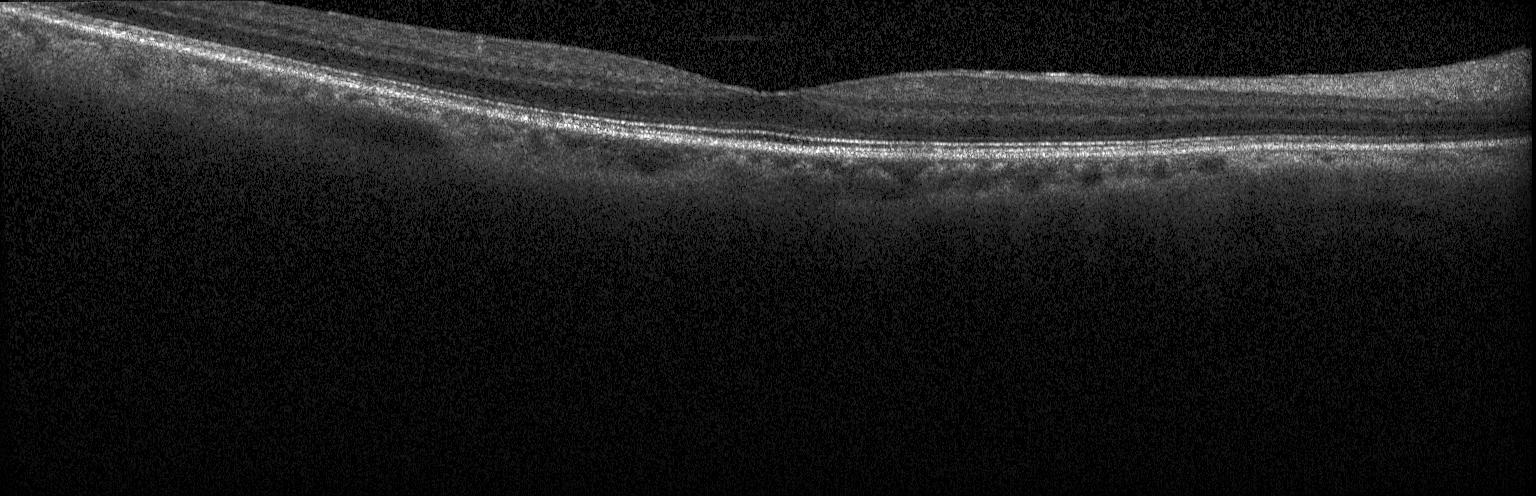

Dx: neither choroidal neovascularization, diabetic macular edema, nor drusen.